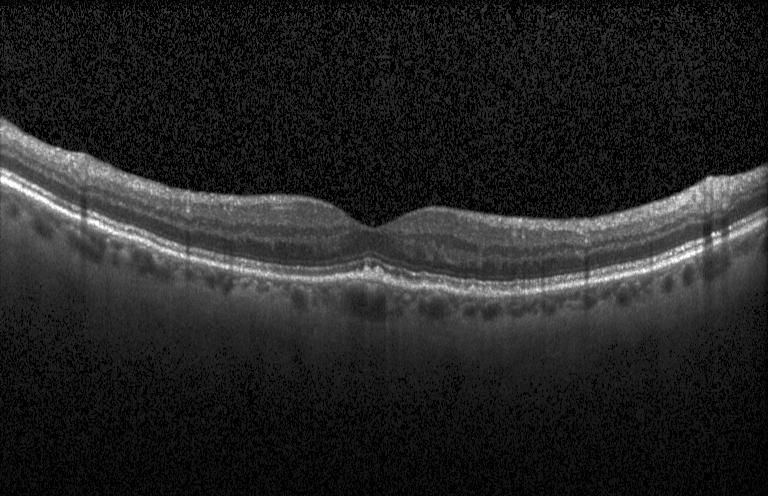
OCT line scan
Finding: sub-RPE drusenoid deposits.